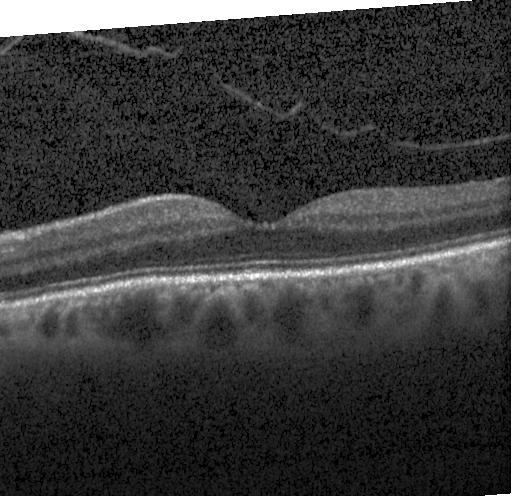 SD-OCT. Retinal OCT B-scan. Fovea-centered. Instrument: Heidelberg Spectralis — This B-scan demonstrates no choroidal neovascularization, no diabetic macular edema, and no drusen.